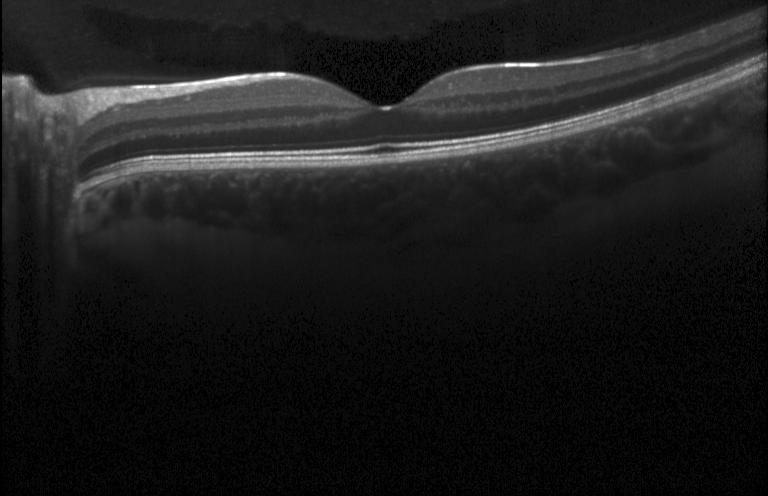
OCT B-scan showing no choroidal neovascularization, diabetic macular edema, or drusen.